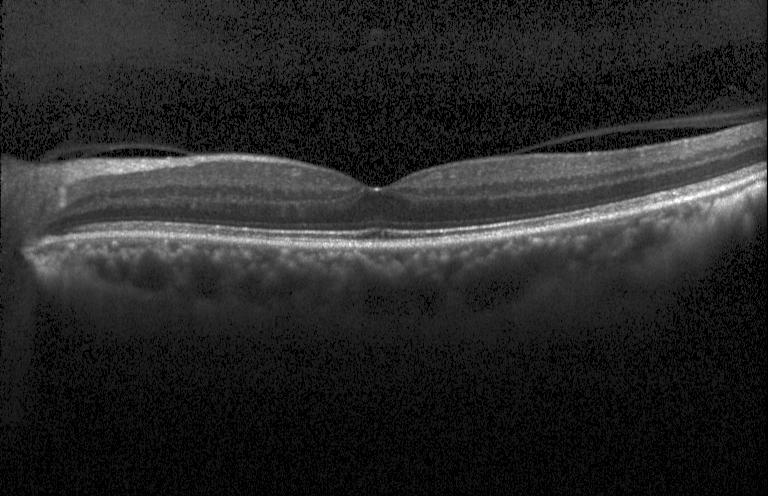

Diagnosis: no choroidal neovascularization, no diabetic macular edema, and no drusen.